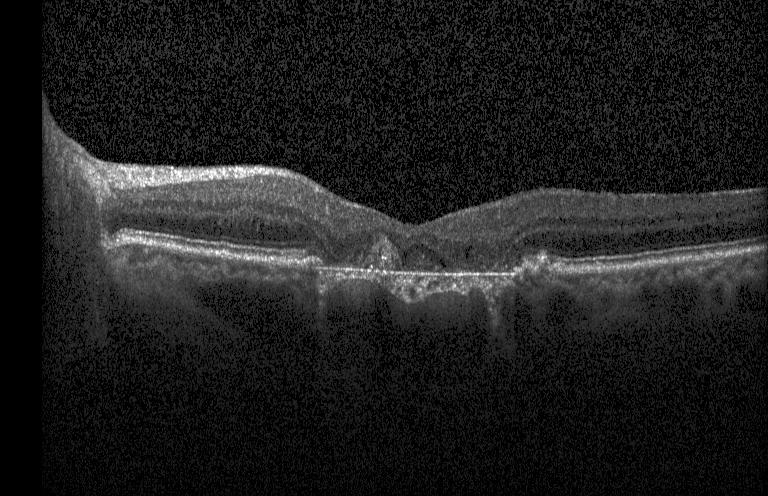
Retinal OCT cross-section. The scan shows choroidal neovascularization (CNV).